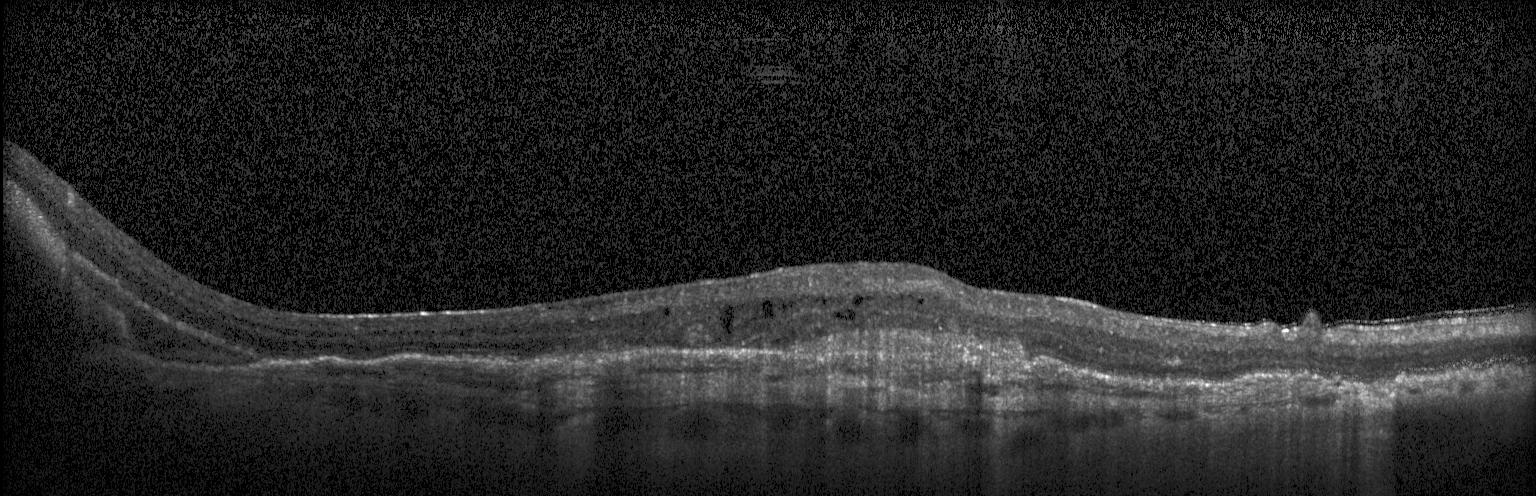

Macular scan. Heidelberg Spectralis OCT system. Retinal OCT B-scan — Assessment: a choroidal neovascular membrane.